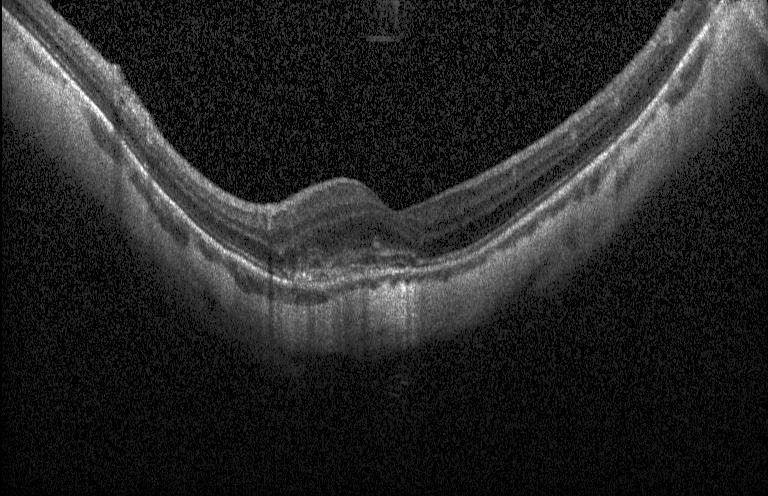

The scan shows CNV.